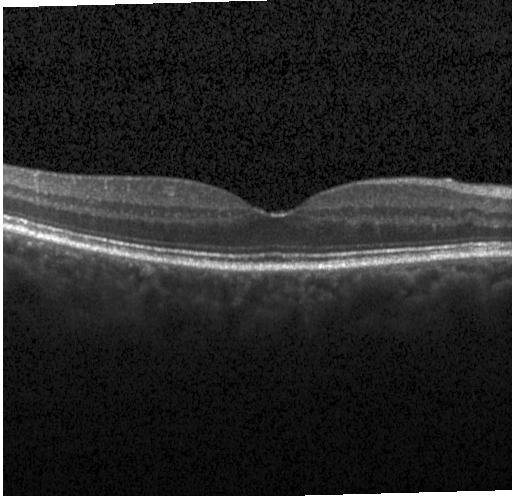
Optical coherence tomography B-scan. Macular scan. Dx: no CNV, no DME, and no drusen.